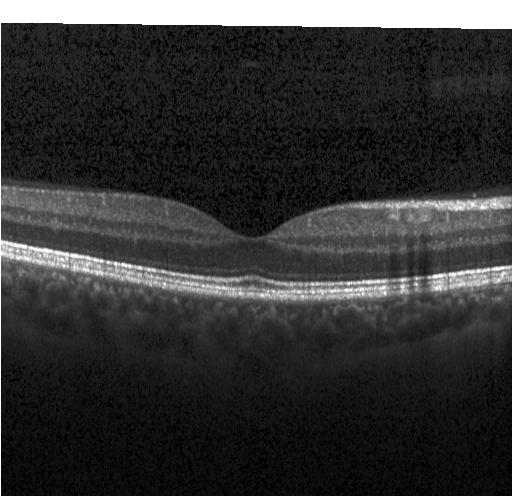

Centered on the fovea · retinal OCT cross-section. Diagnosis: neither choroidal neovascularization, diabetic macular edema, nor drusen.